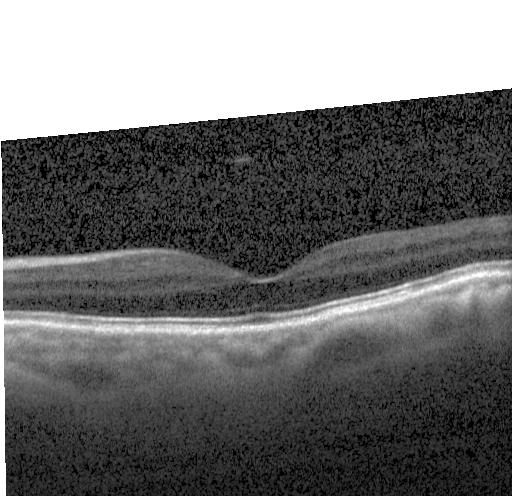

Retinal OCT B-scan. OCT finding: neither choroidal neovascularization, diabetic macular edema, nor drusen.